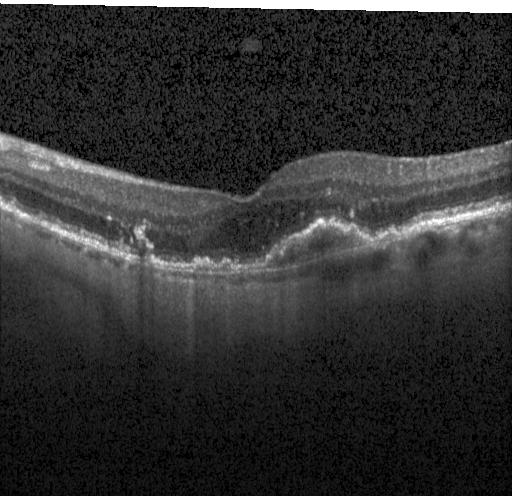
This B-scan demonstrates CNV.